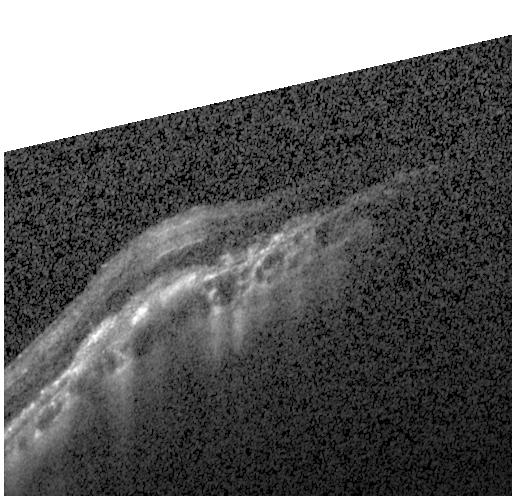
Retinal OCT cross-section showing choroidal neovascularization.